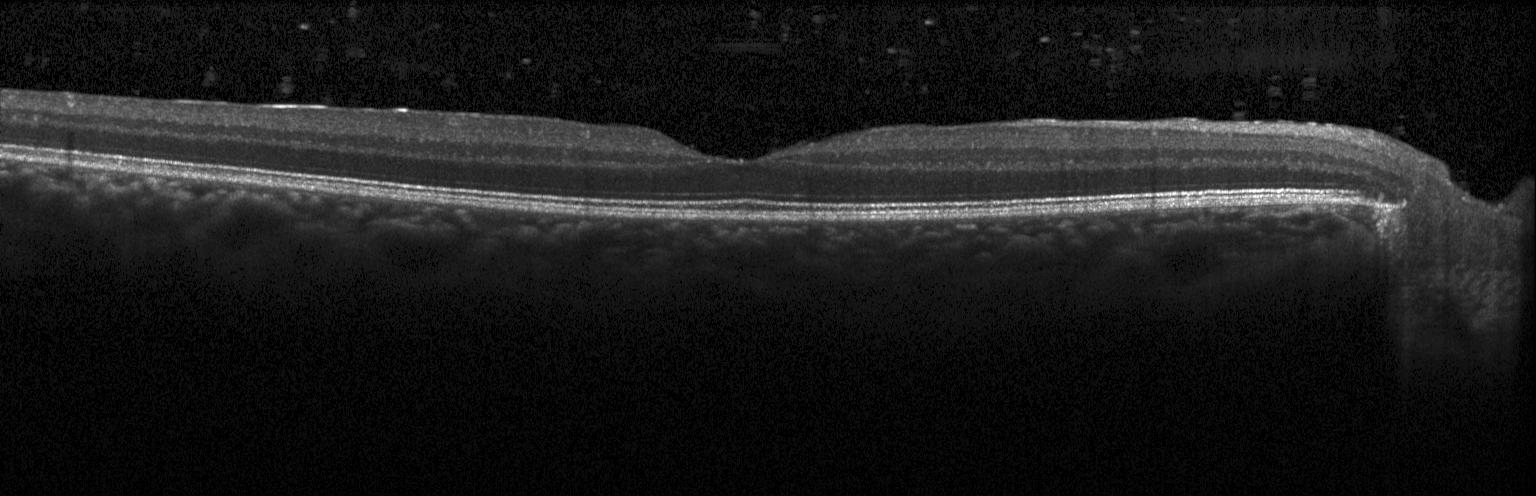

Spectral-domain OCT · retinal OCT B-scan — Dx: no evidence of choroidal neovascularization, diabetic macular edema, or drusen.